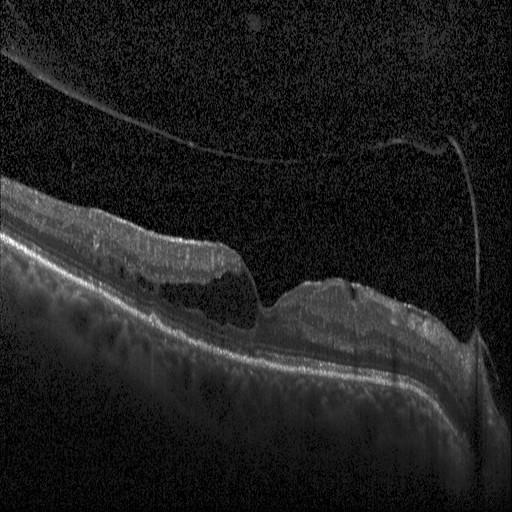

Diagnosis: diabetic macular edema.